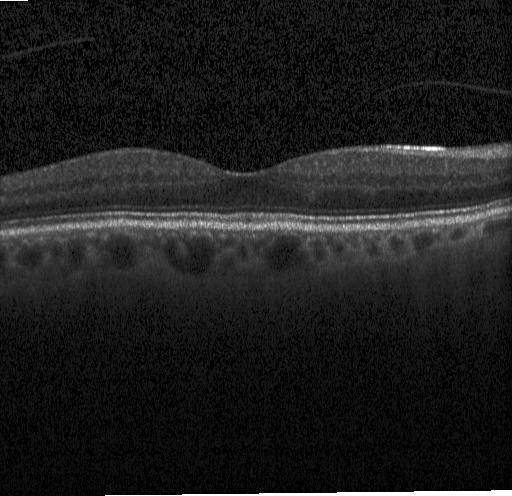 Through the macula. Heidelberg Spectralis. Optical coherence tomography scan
Diagnosis: neither choroidal neovascularization, diabetic macular edema, nor drusen.